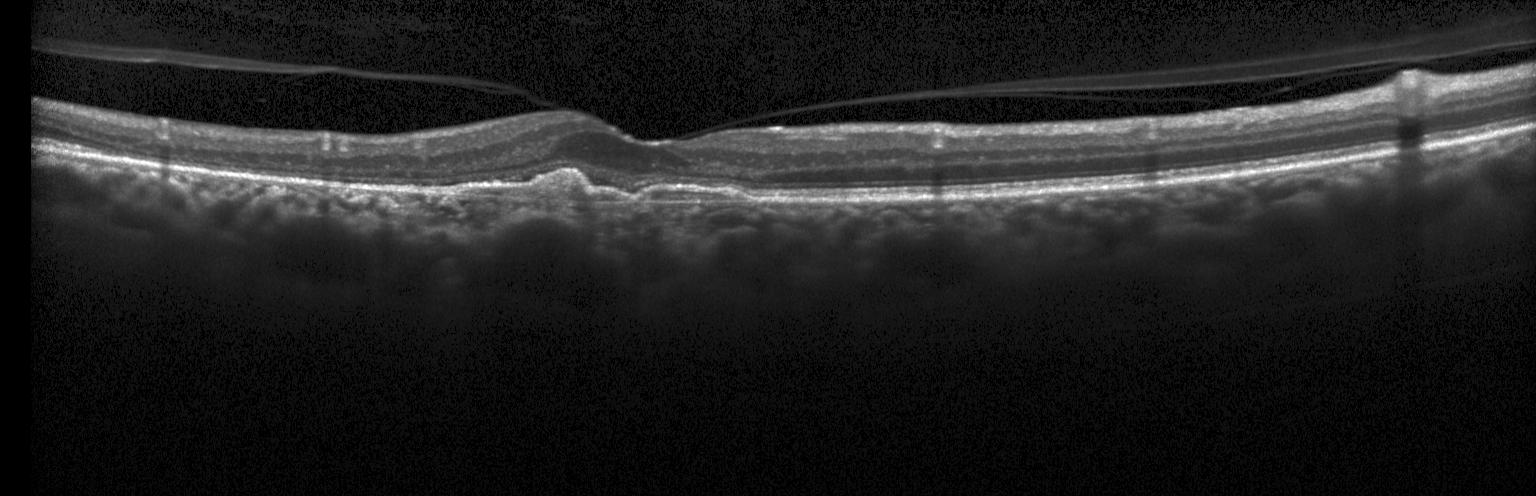
Macular OCT: choroidal neovascularization (CNV).